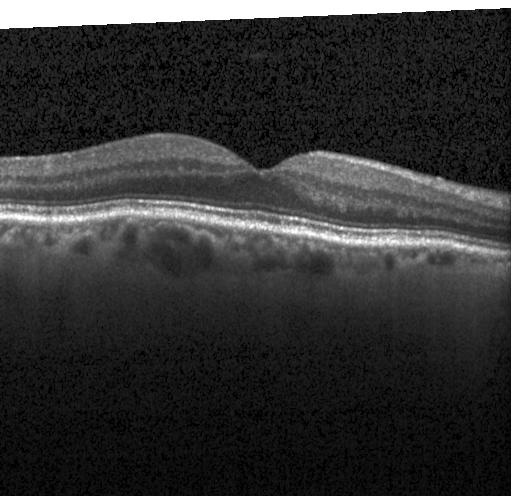 OCT finding: no CNV, no DME, and no drusen.